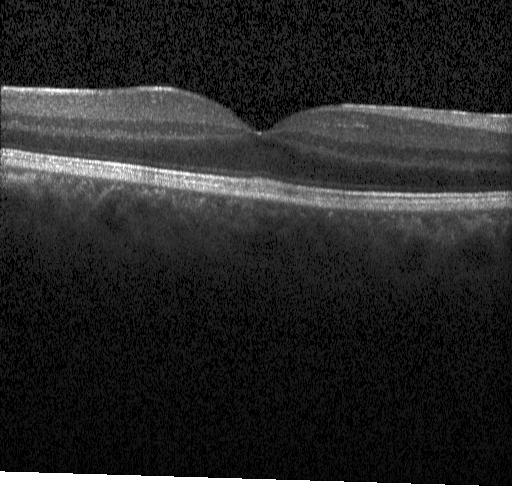 Retinal OCT cross-section showing no evidence of choroidal neovascularization, diabetic macular edema, or drusen.